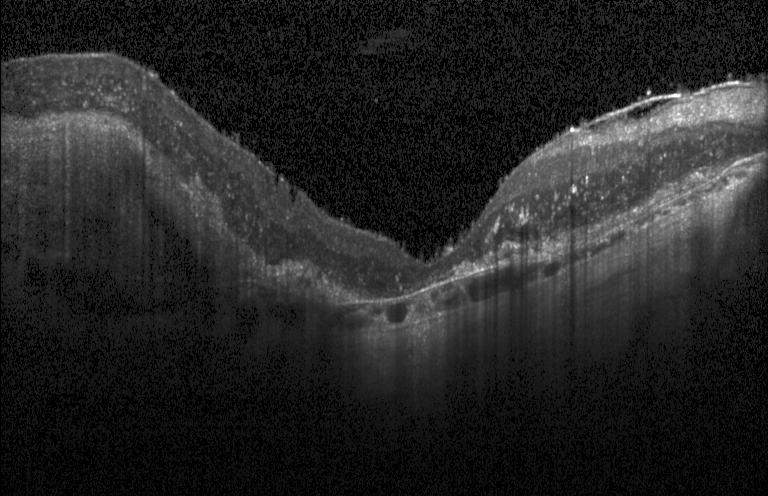

Spectral-domain optical coherence tomography, OCT line scan — Dx: choroidal neovascularization (CNV).